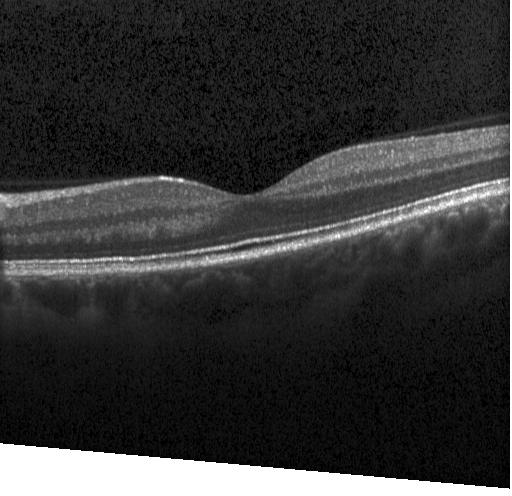
Retinal OCT B-scan — OCT finding: no CNV, DME, or drusen.